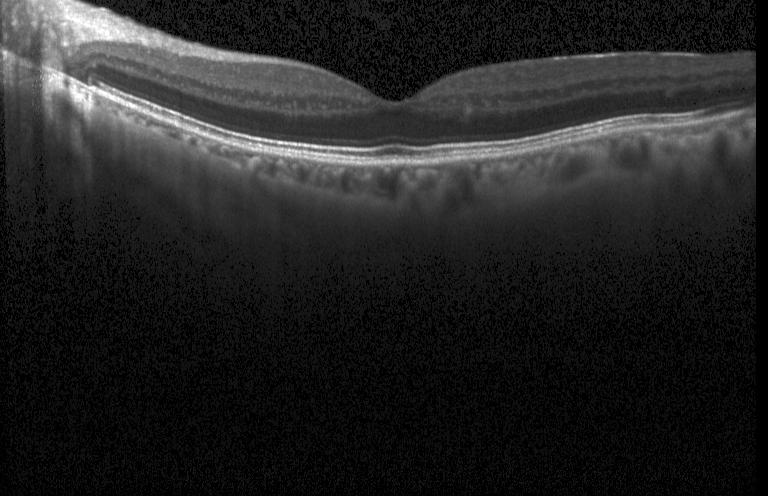 OCT B-scan · Heidelberg Spectralis OCT system · through the macula · SD-OCT
The scan shows neither choroidal neovascularization, diabetic macular edema, nor drusen.